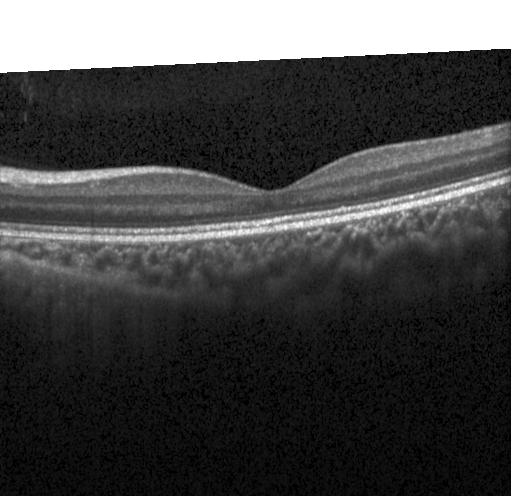
Heidelberg Spectralis OCT system. SD-OCT. Retinal OCT B-scan. Horizontal scan through the fovea.
OCT finding: no CNV, no DME, and no drusen.